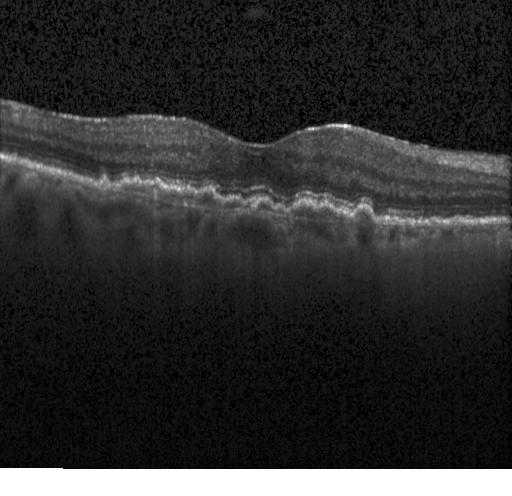
Horizontal scan through the fovea; spectral-domain OCT; instrument: Heidelberg Spectralis; optical coherence tomography B-scan — CNV.